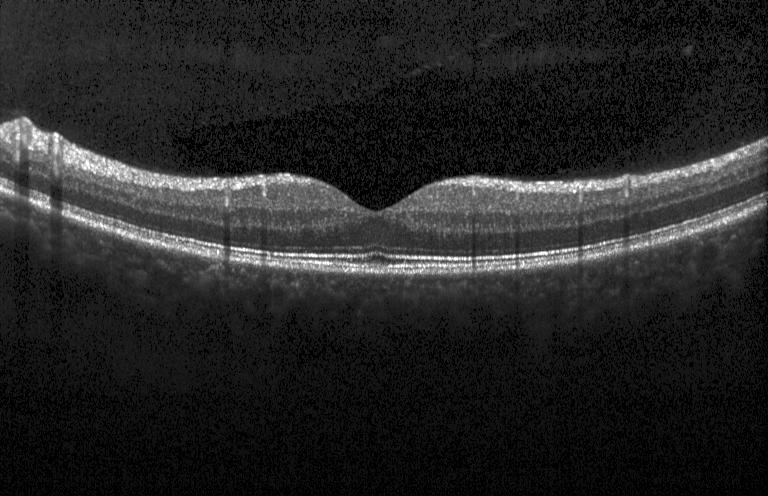 OCT B-scan · horizontal scan through the fovea · spectral-domain OCT · Heidelberg Spectralis
This B-scan demonstrates no choroidal neovascularization, no diabetic macular edema, and no drusen.